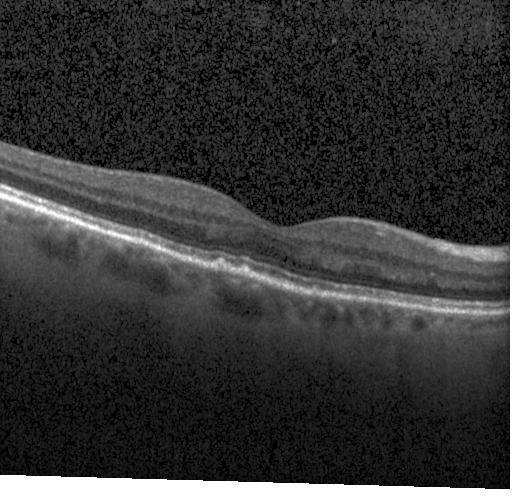

OCT B-scan. SD-OCT. This B-scan demonstrates drusen.